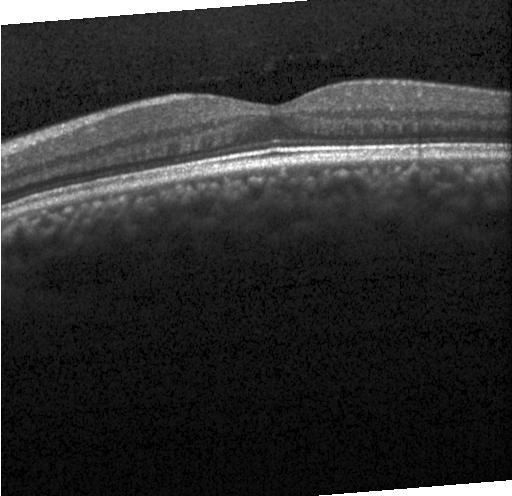

Finding: no CNV, DME, or drusen.